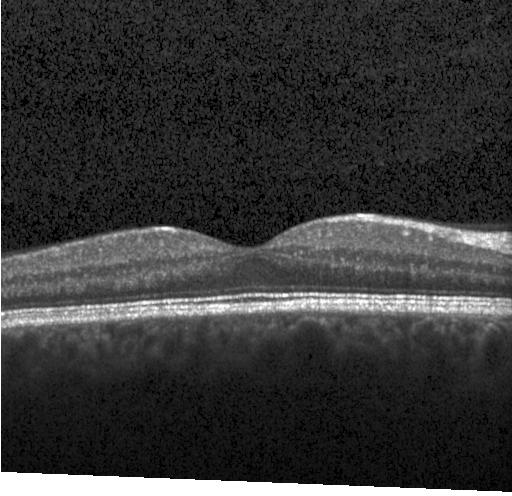 OCT finding: no choroidal neovascularization, no diabetic macular edema, and no drusen.